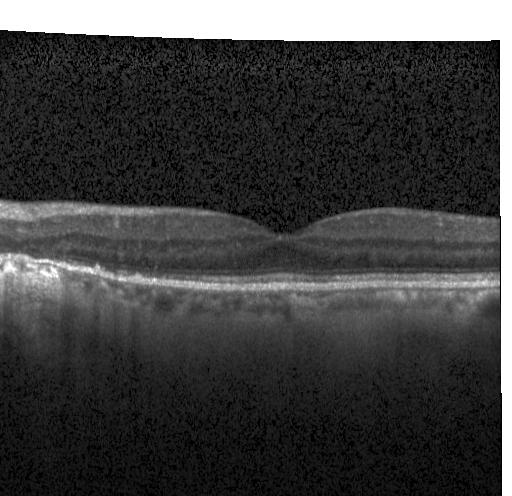

Optical coherence tomography scan.
Impression: neither CNV, DME, nor drusen.